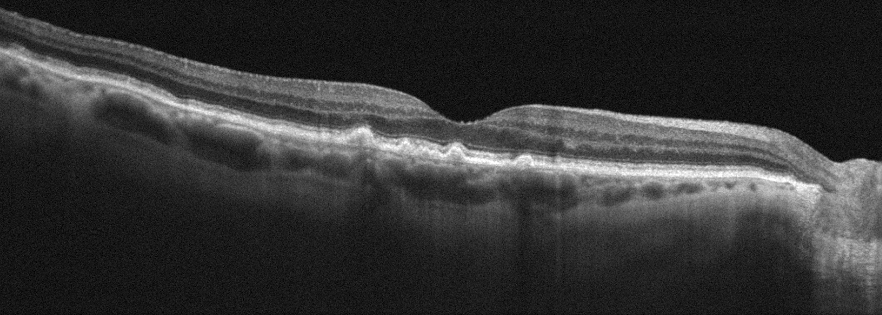 OCT line scan · oculus dexter.
OCT finding: age-related macular degeneration (AMD).